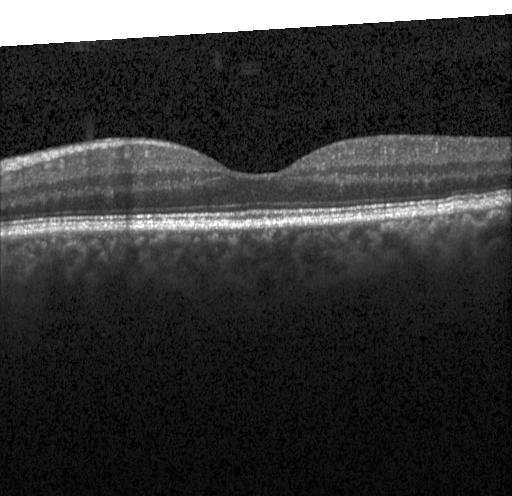 Optical coherence tomography B-scan. Through the macula. Heidelberg Spectralis. Spectral-domain OCT. OCT finding: no CNV, no DME, and no drusen.